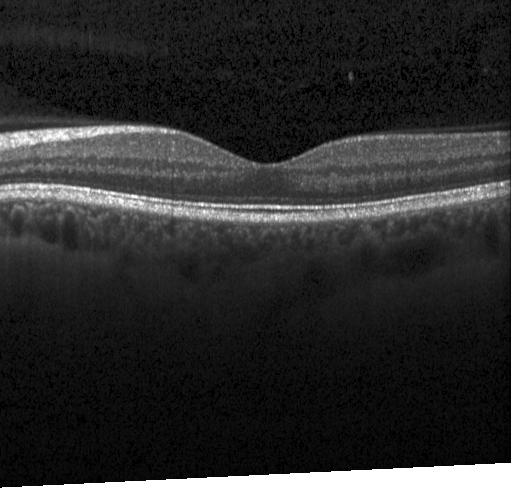
Macular scan, retinal OCT cross-section, acquired on a Heidelberg Spectralis, spectral-domain optical coherence tomography — Finding: no choroidal neovascularization, no diabetic macular edema, and no drusen.